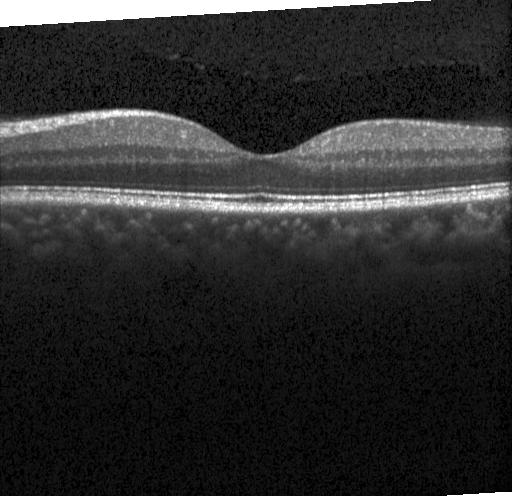
Macular OCT: no evidence of choroidal neovascularization, diabetic macular edema, or drusen.